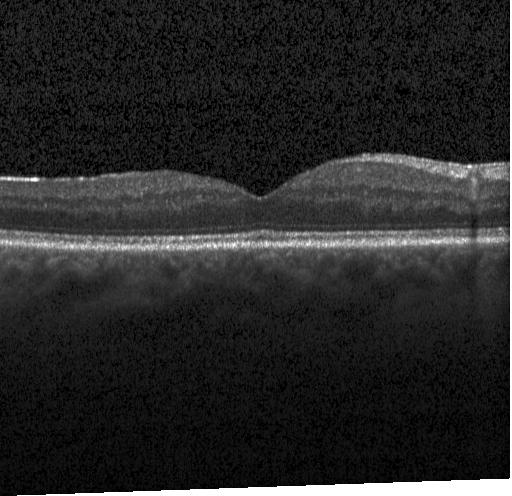 Impression: no choroidal neovascularization, no diabetic macular edema, and no drusen.